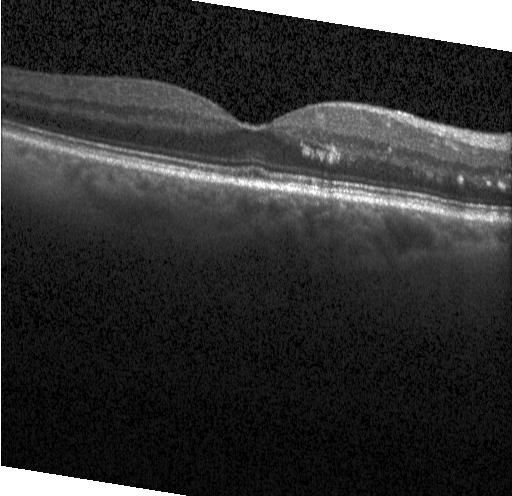 Impression: no evidence of CNV, DME, or drusen.